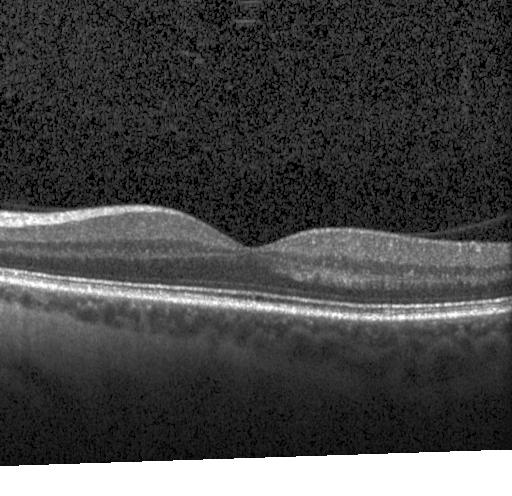
This B-scan demonstrates no CNV, no DME, and no drusen.